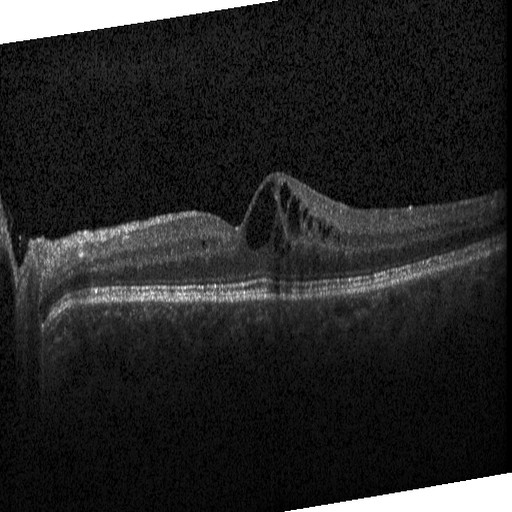 OCT B-scan
OCT finding: diabetic macular edema.